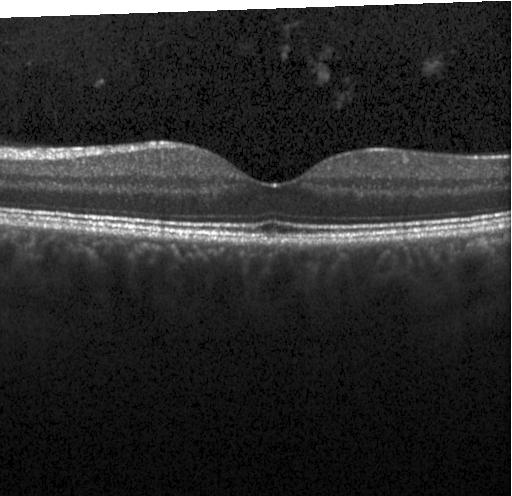 OCT finding: no choroidal neovascularization, diabetic macular edema, or drusen.